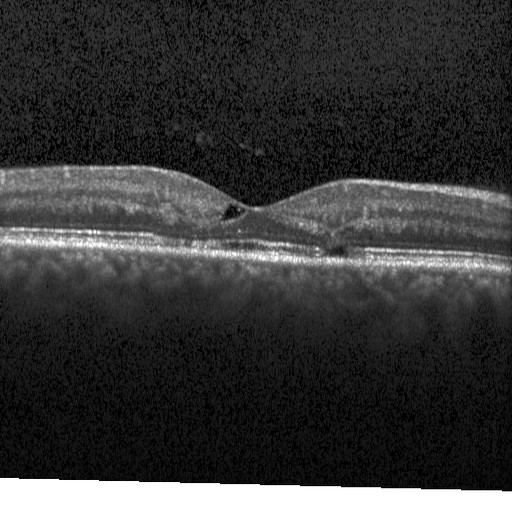
Macular OCT: diabetic macular edema.